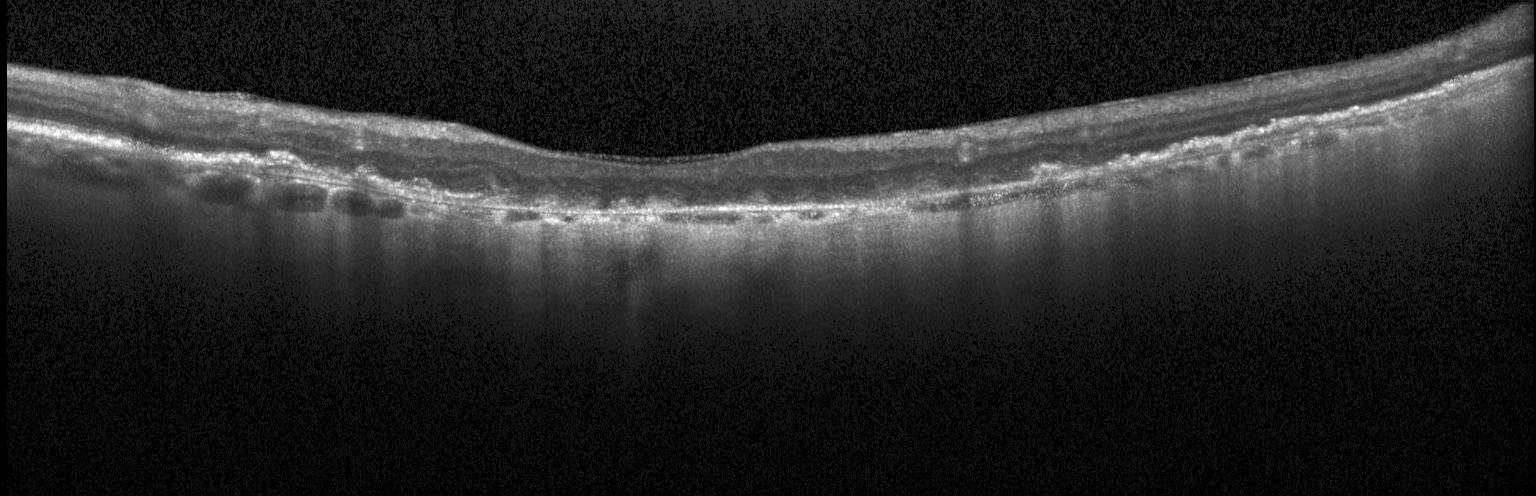

OCT line scan; SD-OCT; fovea-centered — Diagnosis: a choroidal neovascular membrane.